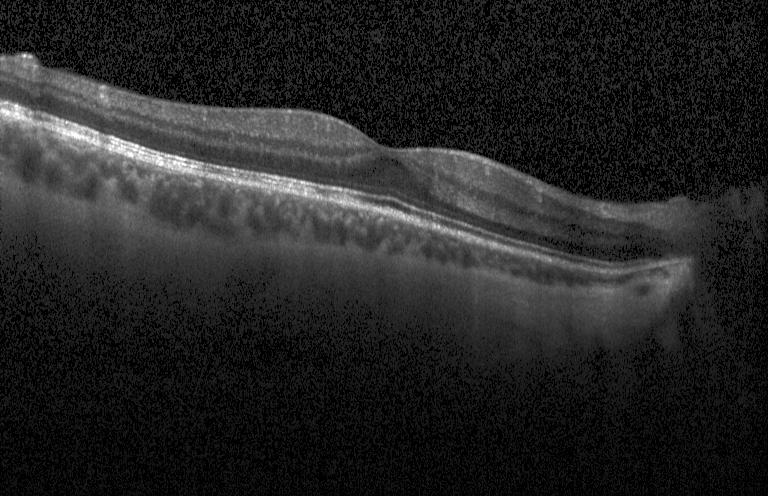
Finding: no choroidal neovascularization, diabetic macular edema, or drusen.